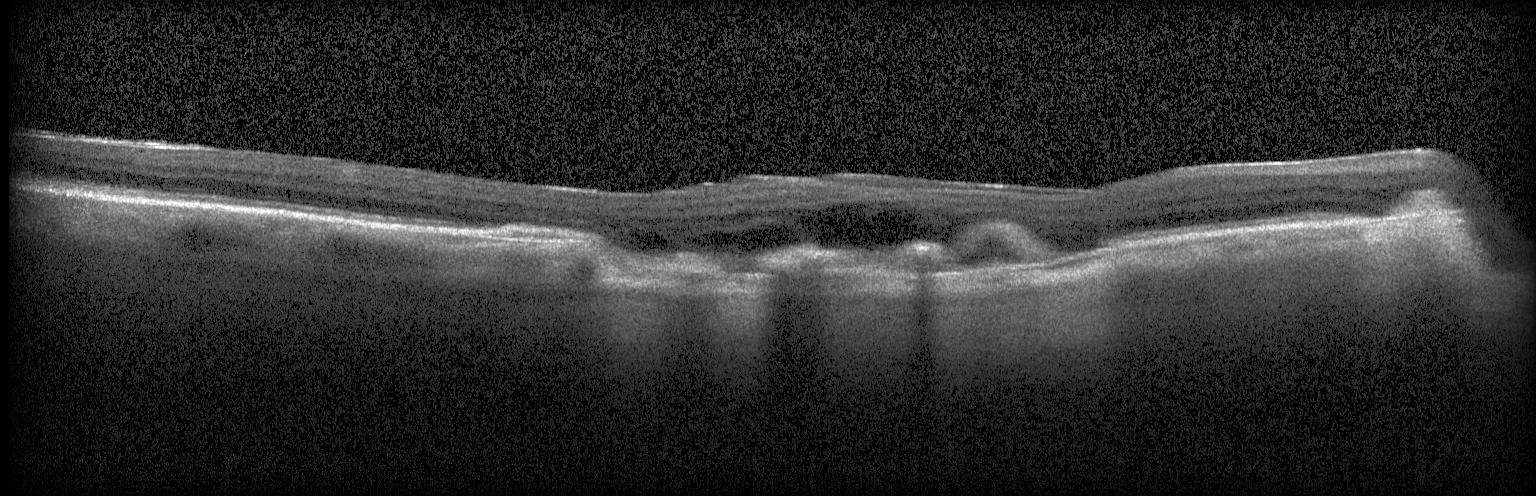
Optical coherence tomography scan · Heidelberg Spectralis OCT system · spectral-domain optical coherence tomography · horizontal scan through the fovea. OCT finding: CNV.